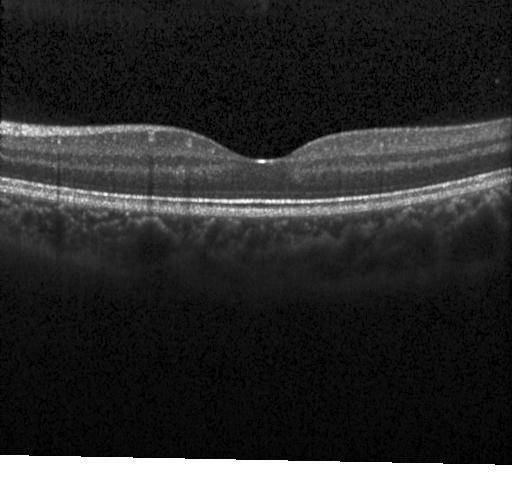 OCT scan showing no choroidal neovascularization, diabetic macular edema, or drusen.